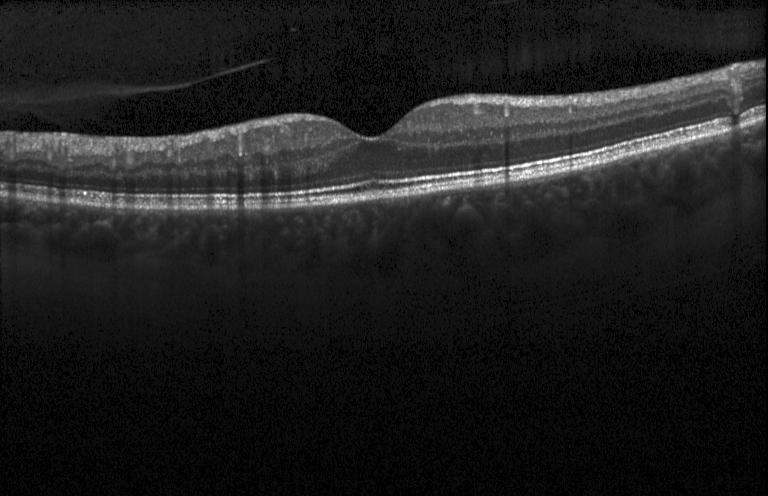
OCT line scan.
Dx: no CNV, no DME, and no drusen.